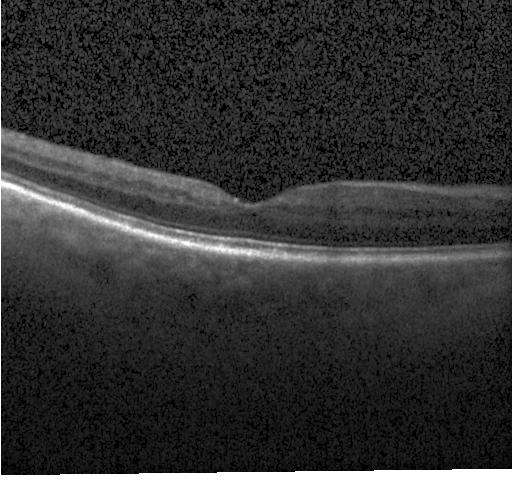
Optical coherence tomography B-scan. Finding: neither choroidal neovascularization, diabetic macular edema, nor drusen.